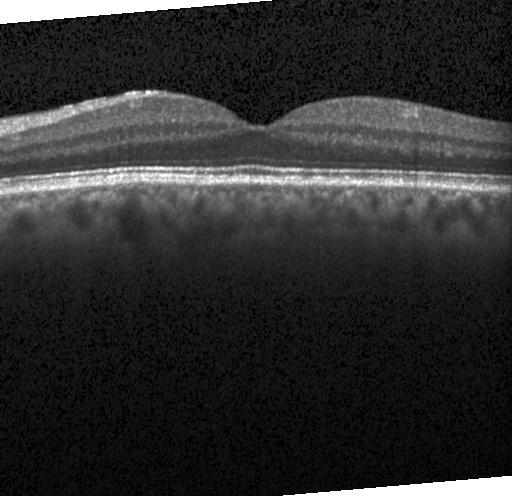
Neither choroidal neovascularization, diabetic macular edema, nor drusen.